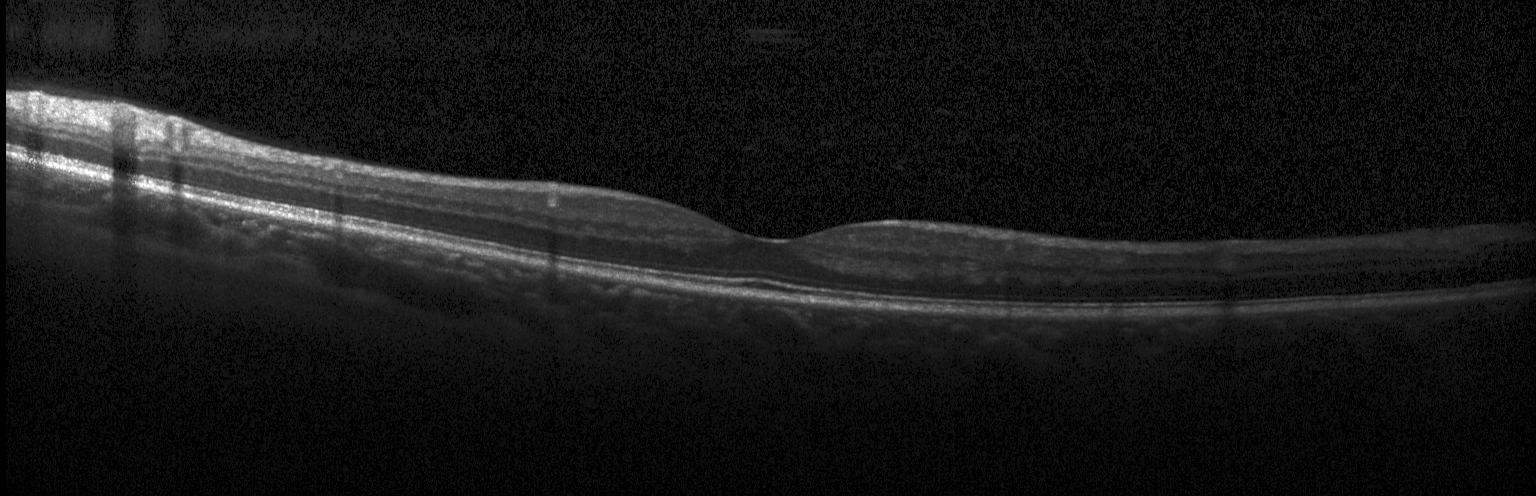 OCT B-scan showing neither choroidal neovascularization, diabetic macular edema, nor drusen.